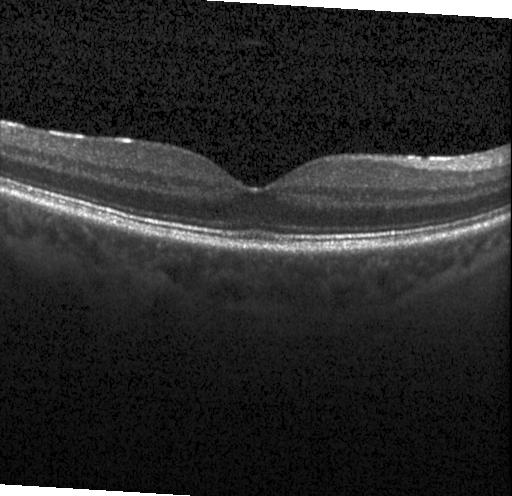
Retinal OCT B-scan; fovea-centered — The scan shows no choroidal neovascularization, diabetic macular edema, or drusen.